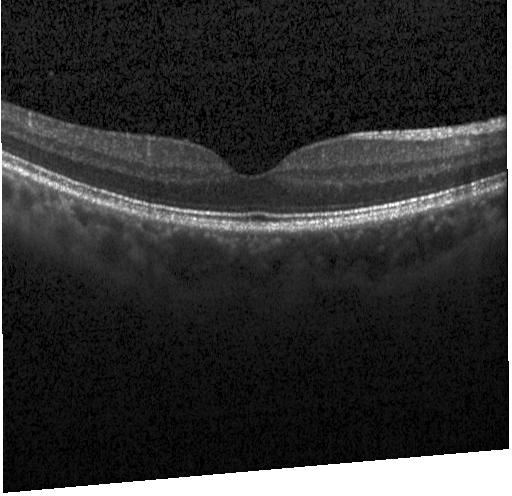

Retinal OCT cross-section · spectral-domain optical coherence tomography
Macular OCT: no CNV, DME, or drusen.